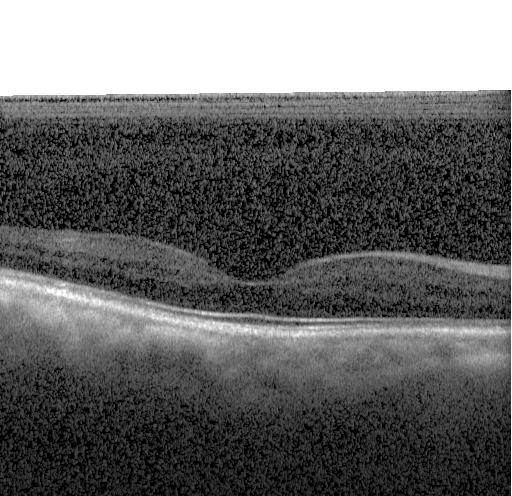 Spectral-domain optical coherence tomography. Horizontal scan through the fovea. Optical coherence tomography scan — The scan shows neither choroidal neovascularization, diabetic macular edema, nor drusen.